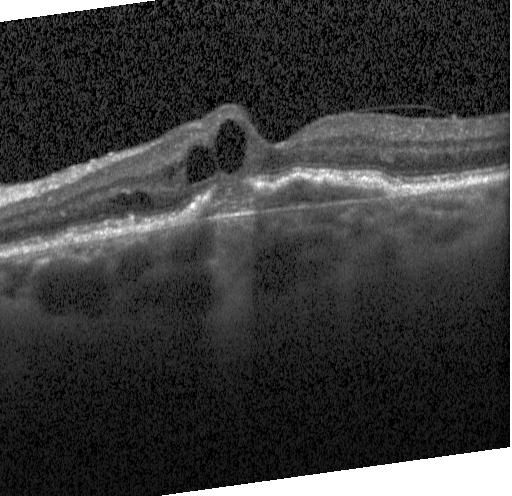 Retinal OCT cross-section, acquired on a Heidelberg Spectralis.
Finding: a choroidal neovascular membrane.